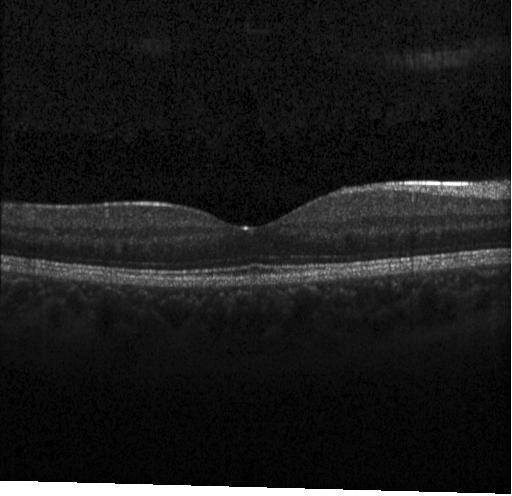

Assessment: neither choroidal neovascularization, diabetic macular edema, nor drusen.